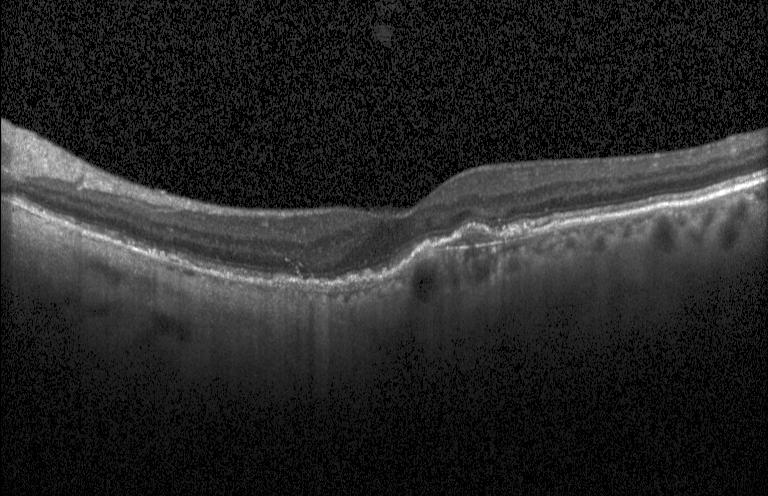 Heidelberg Spectralis OCT system; SD-OCT; retinal OCT cross-section; horizontal scan through the fovea. Dx: CNV.